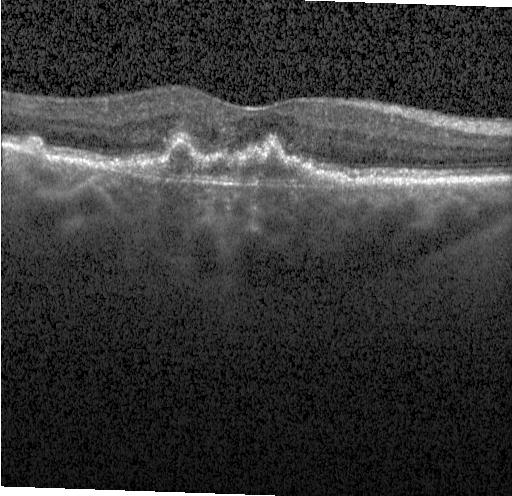
Retinal OCT cross-section — Impression: choroidal neovascularization (CNV).